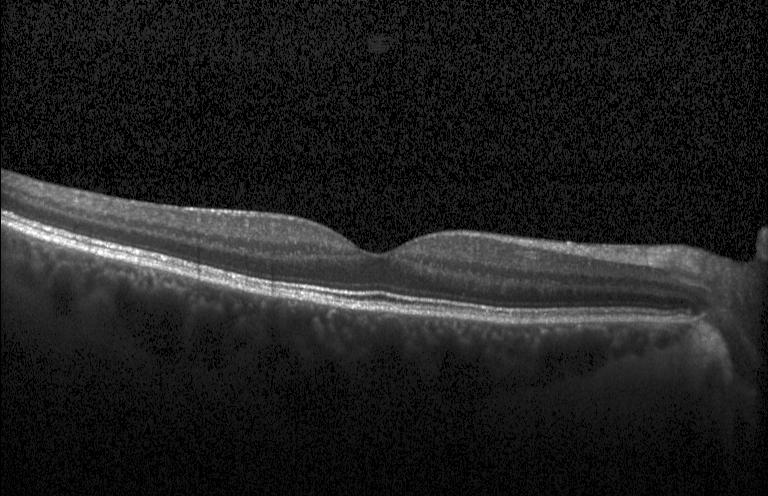 SD-OCT. Through the macula. Instrument: Heidelberg Spectralis. Retinal OCT cross-section.
No CNV, no DME, and no drusen.